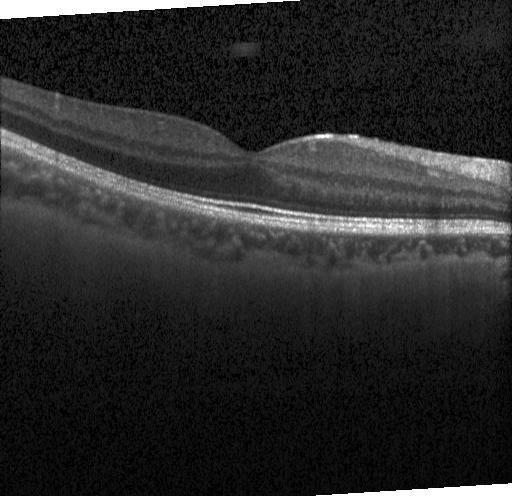 Macular OCT demonstrating no choroidal neovascularization, diabetic macular edema, or drusen.